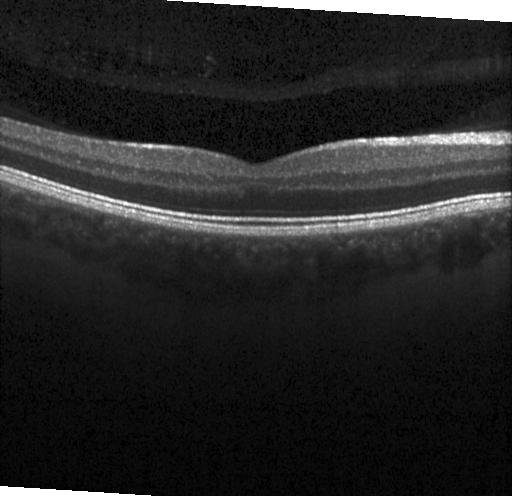

Optical coherence tomography scan
This B-scan demonstrates neither choroidal neovascularization, diabetic macular edema, nor drusen.